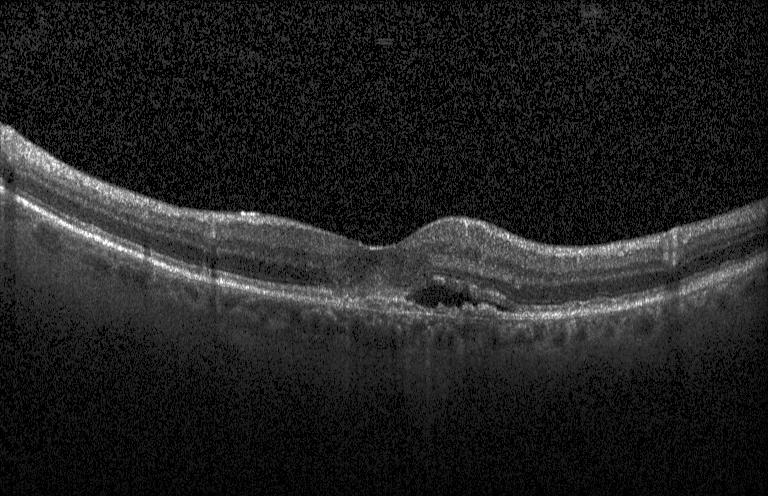
Spectral-domain optical coherence tomography, optical coherence tomography B-scan — Finding: a choroidal neovascular membrane.